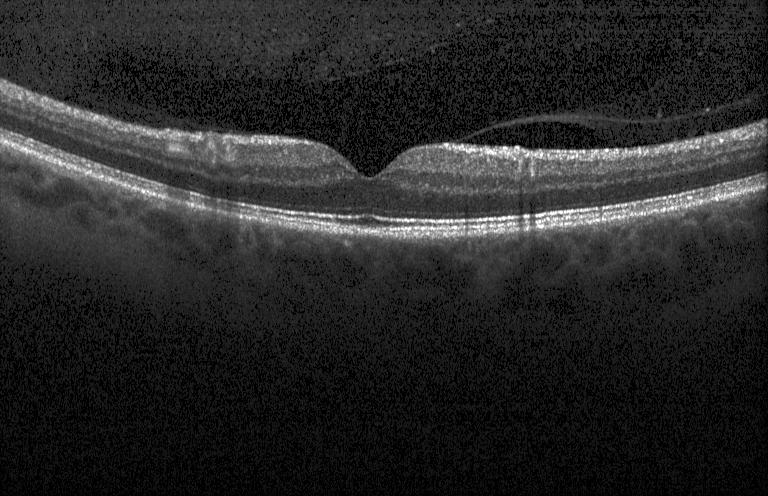 Spectral-domain OCT B-scan: no evidence of CNV, DME, or drusen.